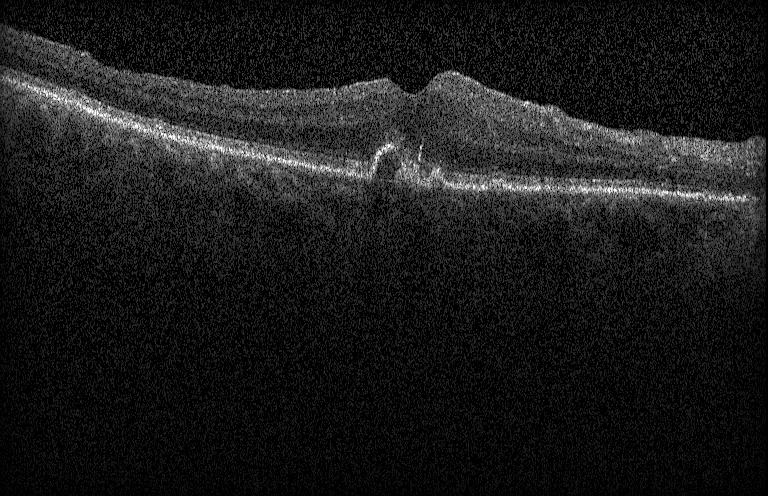

OCT scan showing sub-RPE drusenoid deposits.